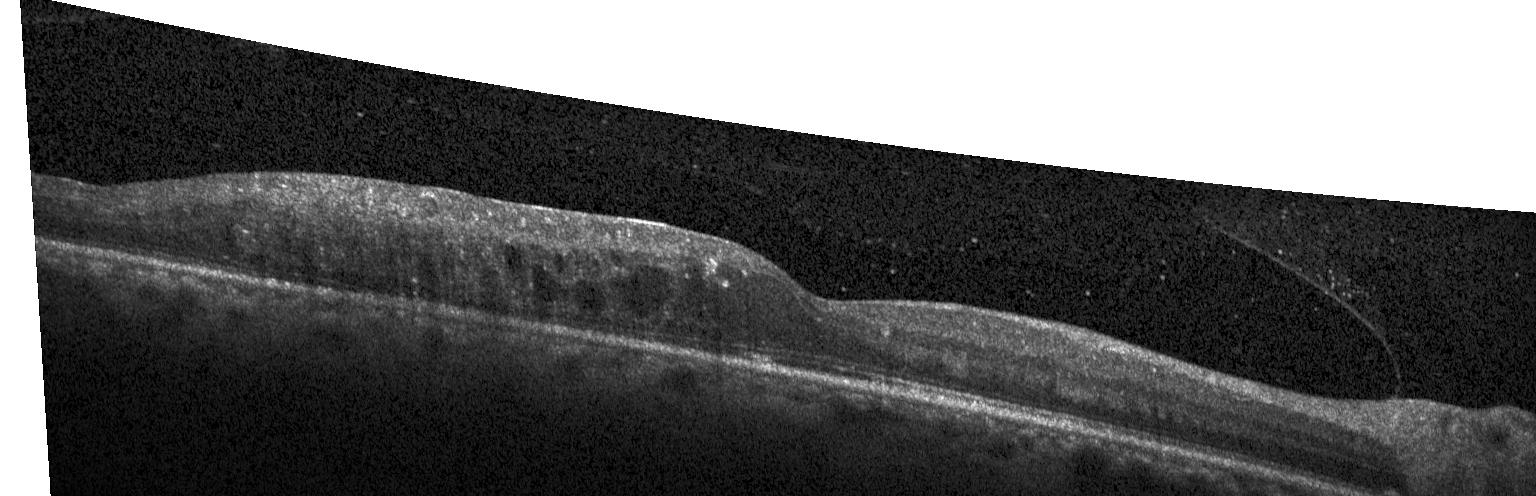

Diagnosis: diabetic macular edema.